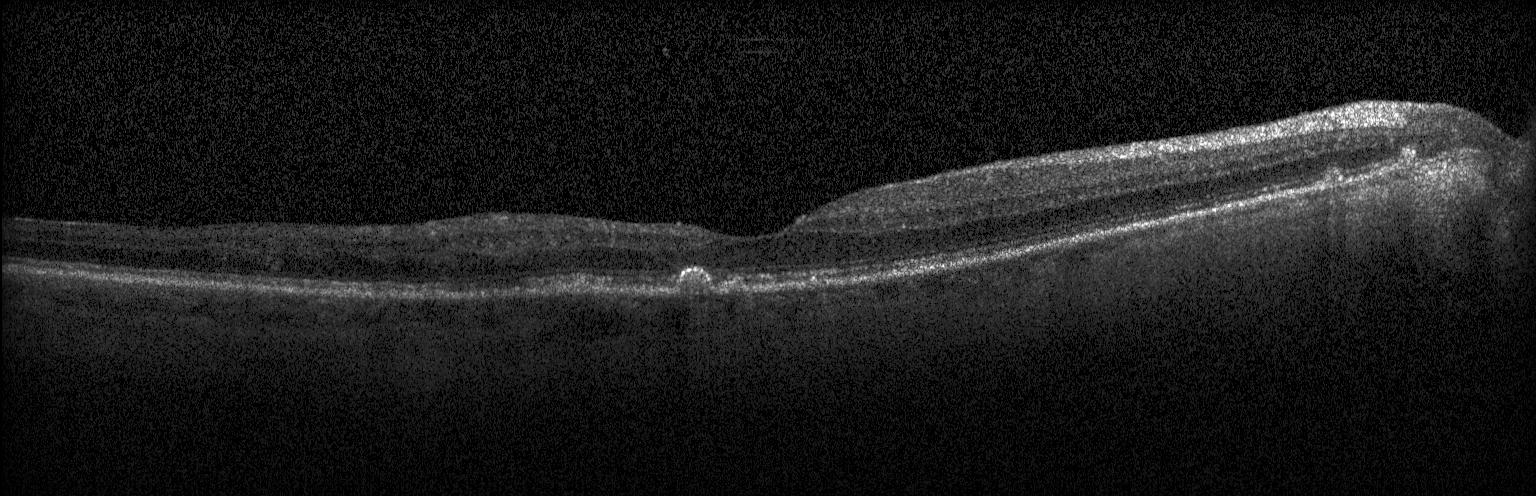

OCT line scan, centered on the fovea — Impression: sub-RPE drusenoid deposits.